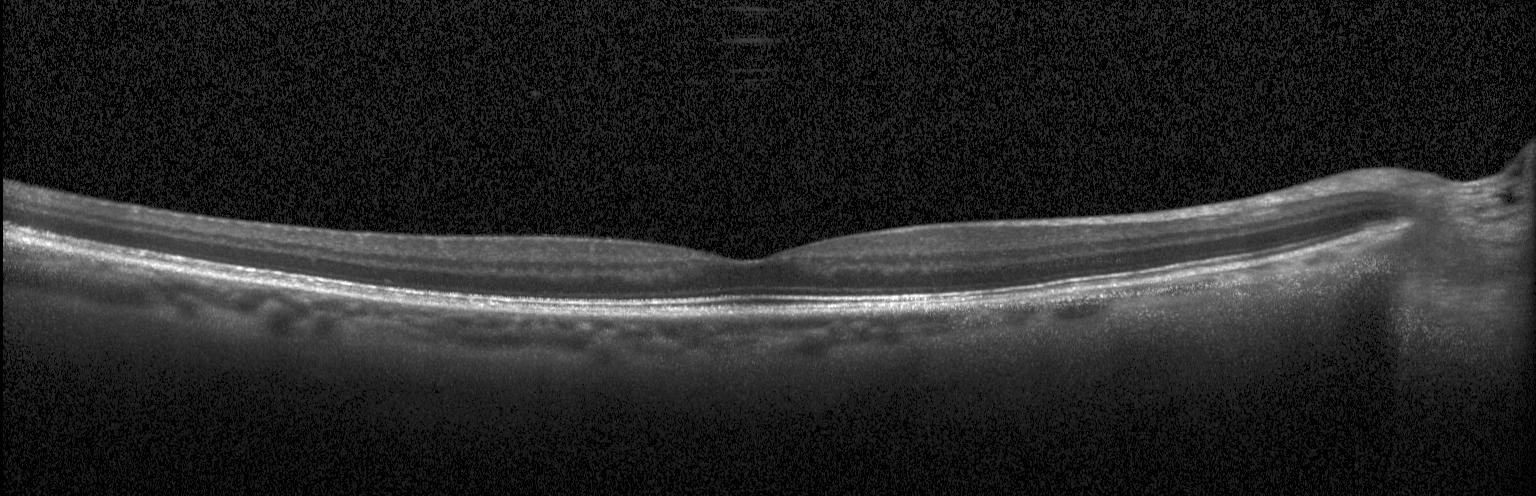 OCT B-scan · acquired on a Heidelberg Spectralis — Diagnosis: neither choroidal neovascularization, diabetic macular edema, nor drusen.